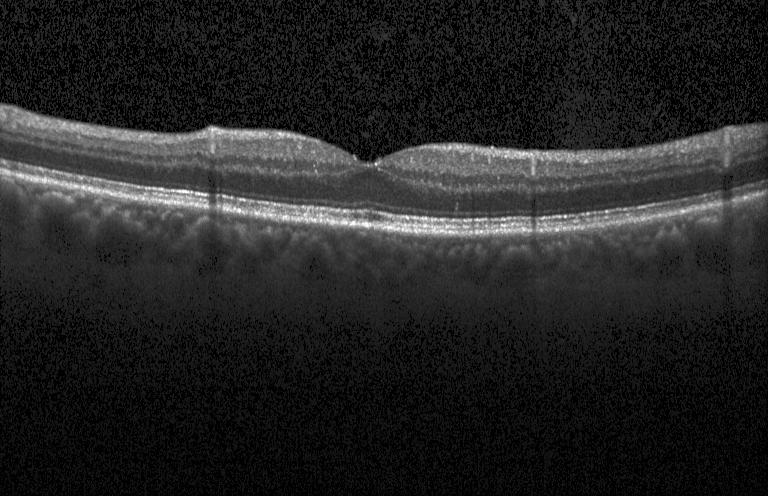 Optical coherence tomography scan. Spectral-domain OCT. Centered on the fovea — Finding: neither choroidal neovascularization, diabetic macular edema, nor drusen.